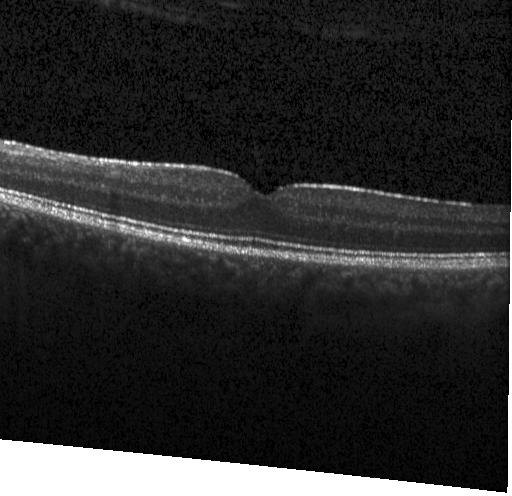
Retinal OCT cross-section. Impression: no evidence of choroidal neovascularization, diabetic macular edema, or drusen.